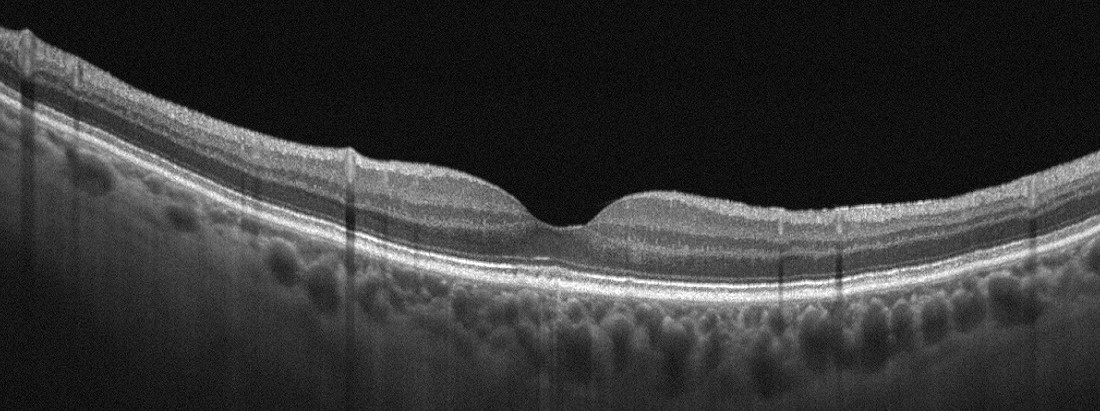
Optovue Avanti RTVue XR, retinal OCT B-scan
Assessment: age-related macular degeneration.